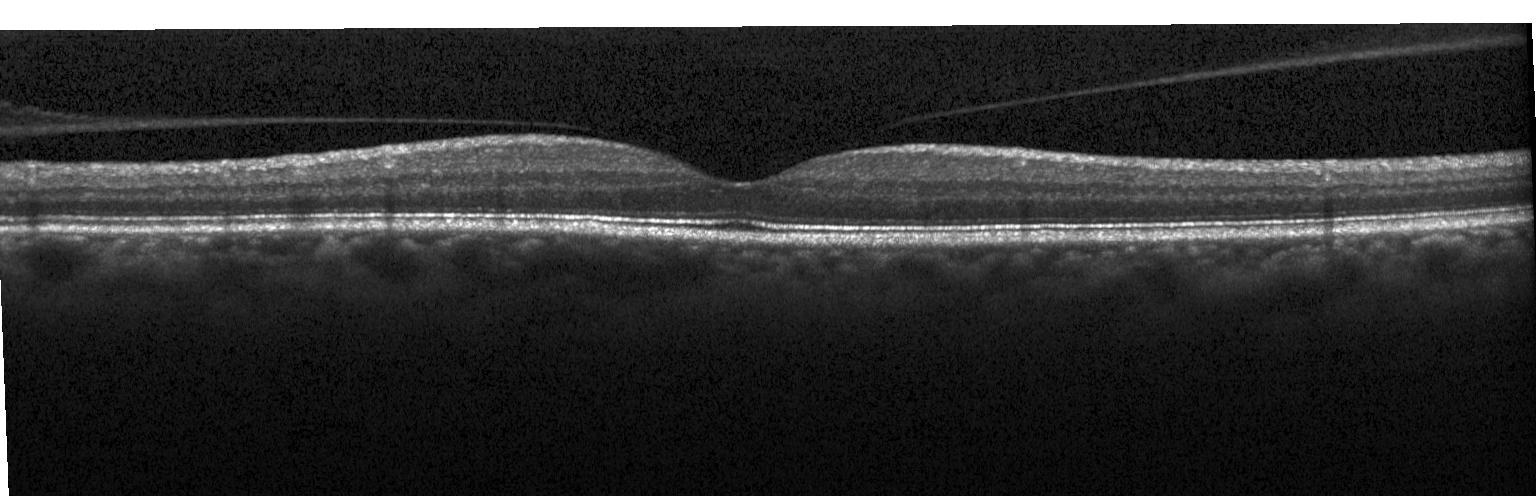
The scan shows neither choroidal neovascularization, diabetic macular edema, nor drusen.